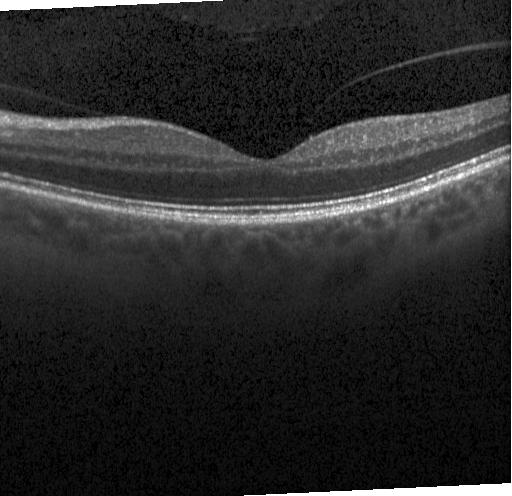
Finding: no choroidal neovascularization, no diabetic macular edema, and no drusen.